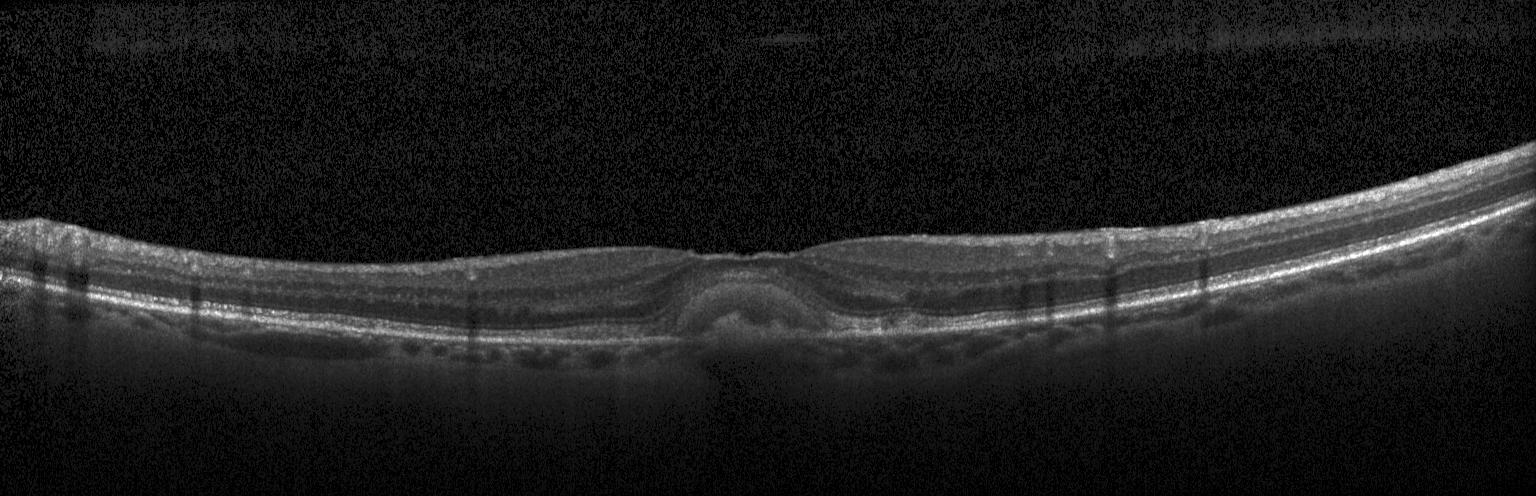
Impression: a choroidal neovascular membrane.